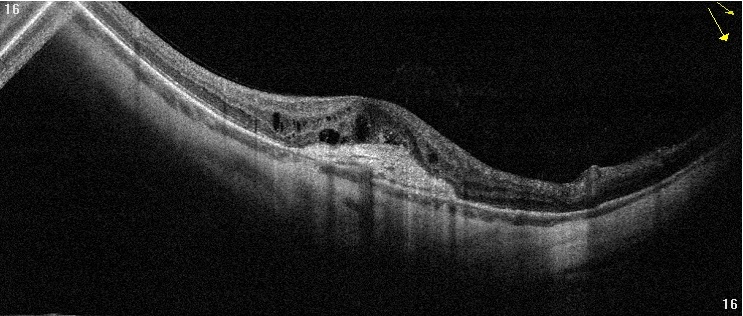
Fovea-centered. Optovue Avanti RTVue XR. Retinal OCT B-scan — Finding: age-related macular degeneration (AMD).